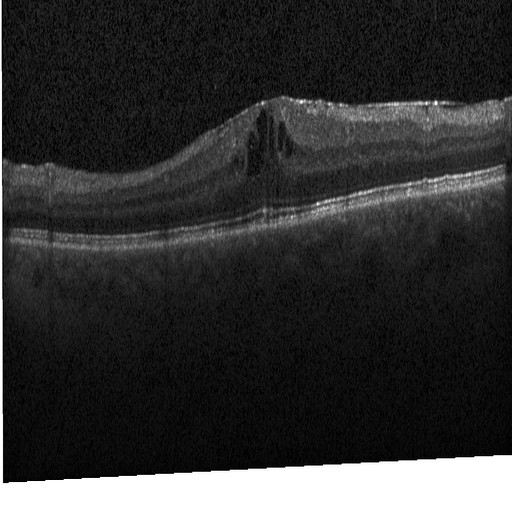
OCT line scan.
This B-scan demonstrates diabetic macular edema (DME).